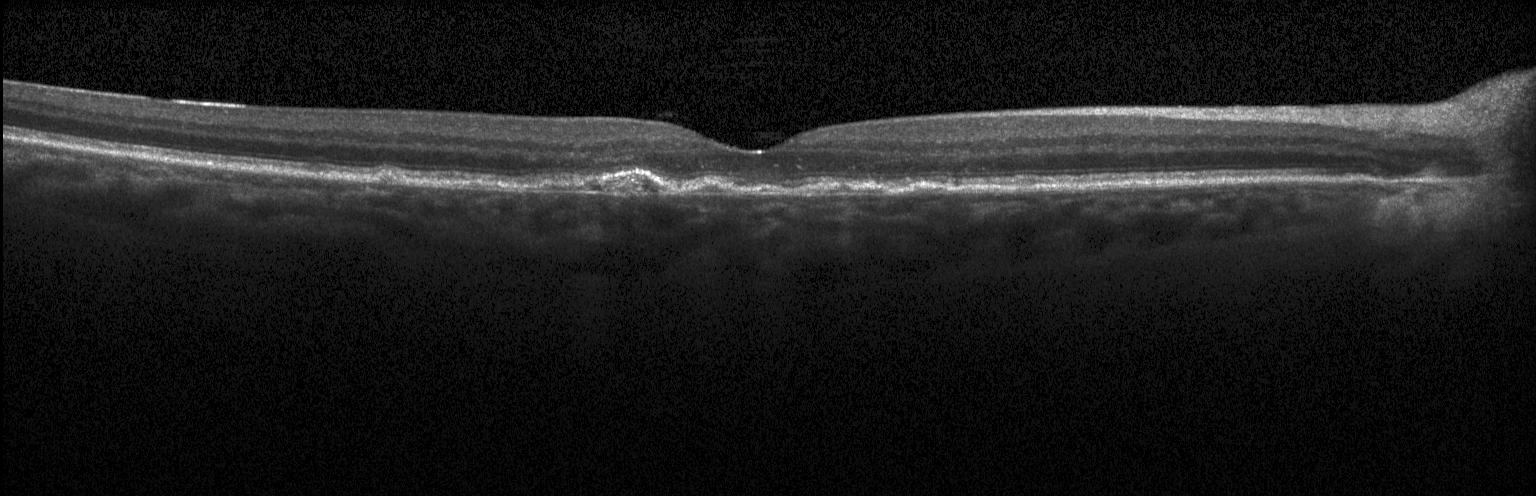 Diagnosis: a choroidal neovascular membrane.